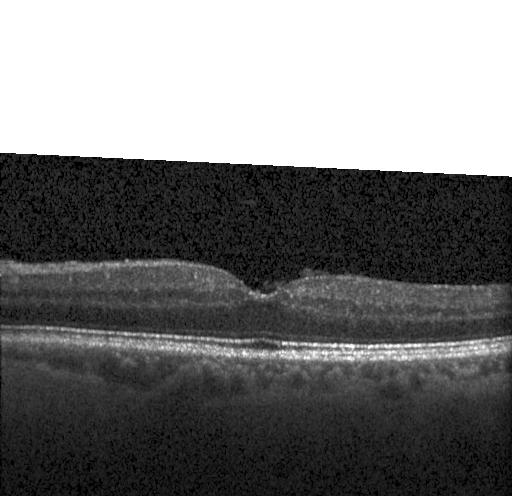 Macular OCT demonstrating no CNV, no DME, and no drusen.